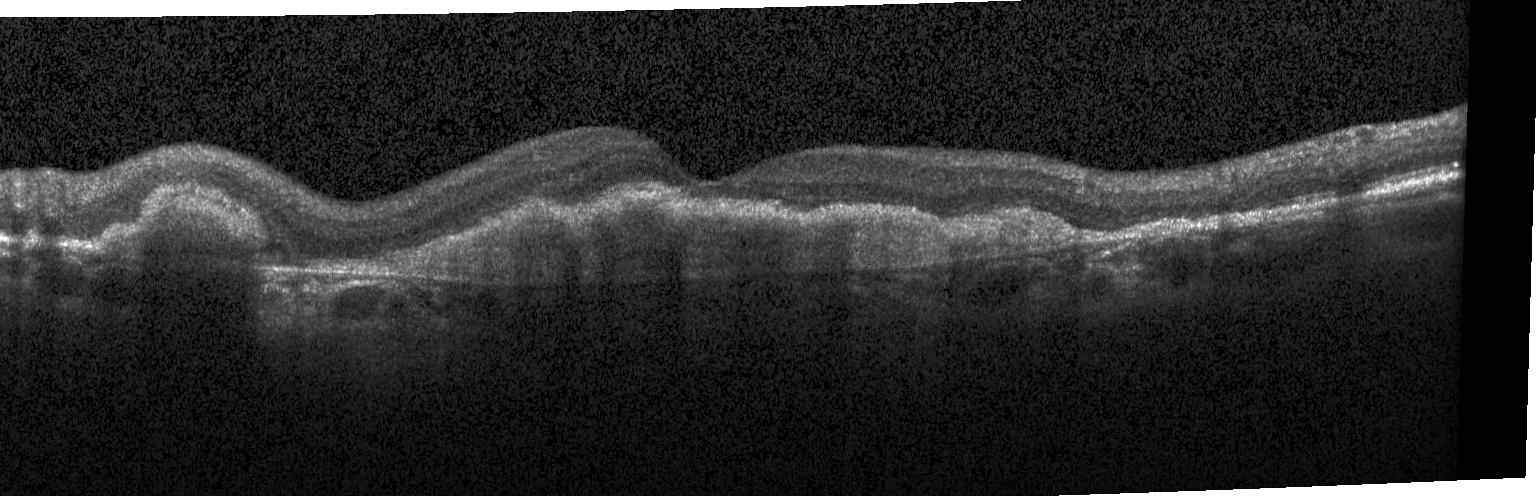 Finding: a choroidal neovascular membrane.